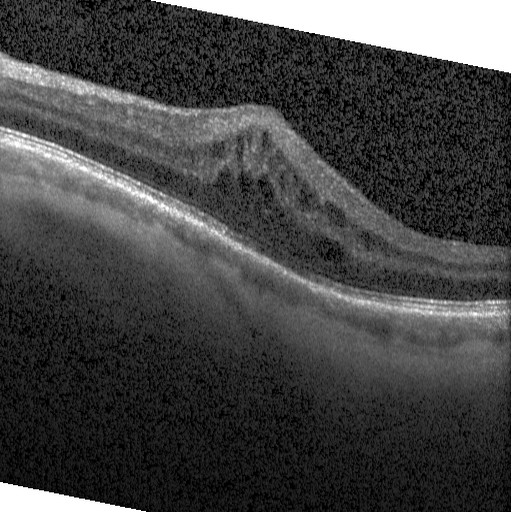

OCT line scan. Diabetic macular edema (DME).